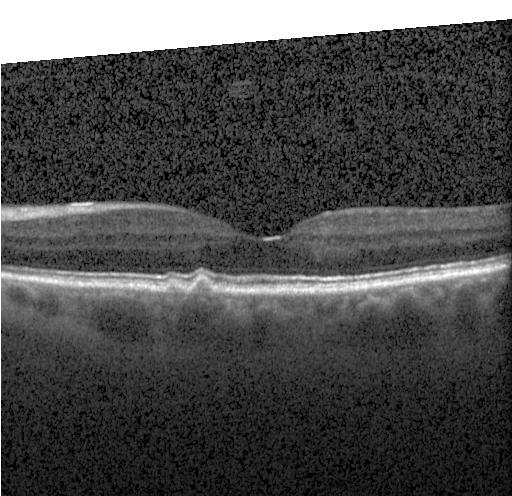
OCT scan showing sub-RPE drusenoid deposits.